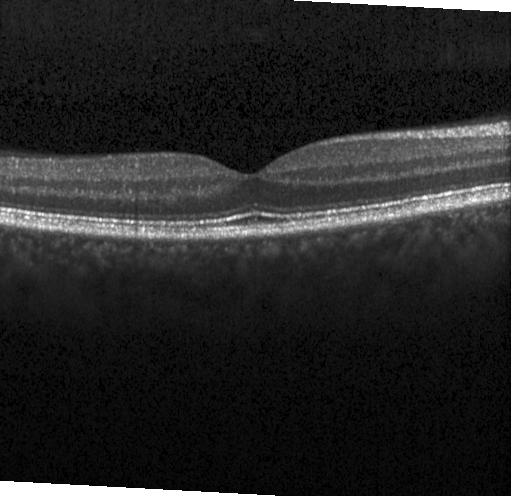

OCT B-scan. Centered on the fovea. Spectral-domain OCT
OCT finding: neither choroidal neovascularization, diabetic macular edema, nor drusen.